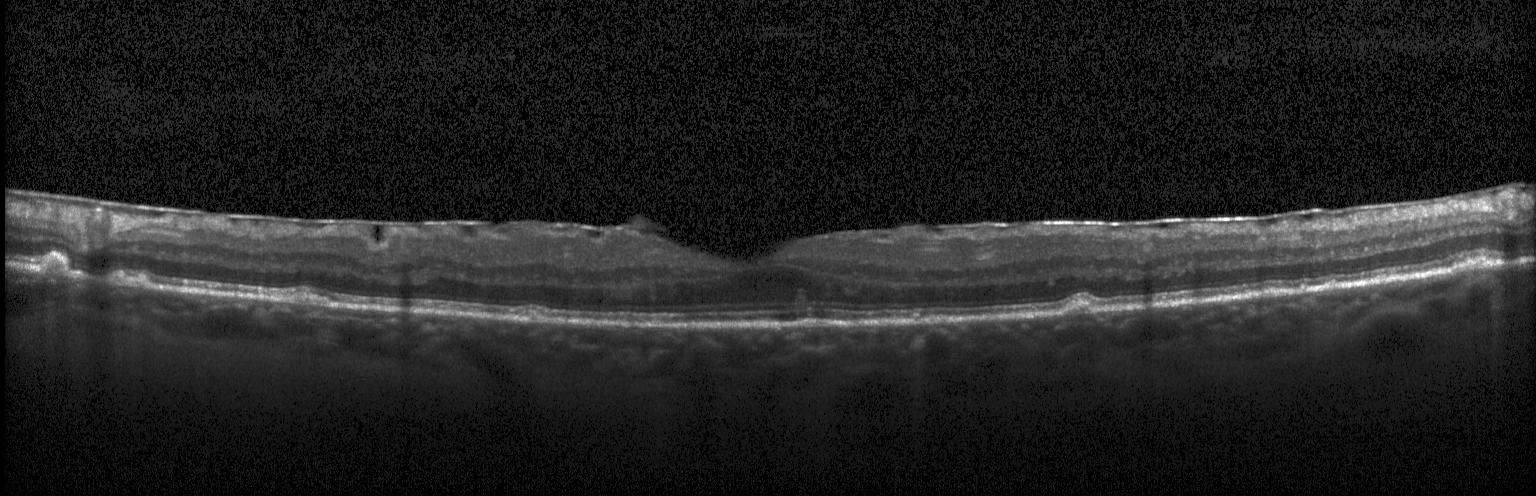 Heidelberg Spectralis OCT system, optical coherence tomography B-scan, spectral-domain optical coherence tomography. Diagnosis: multiple drusen.